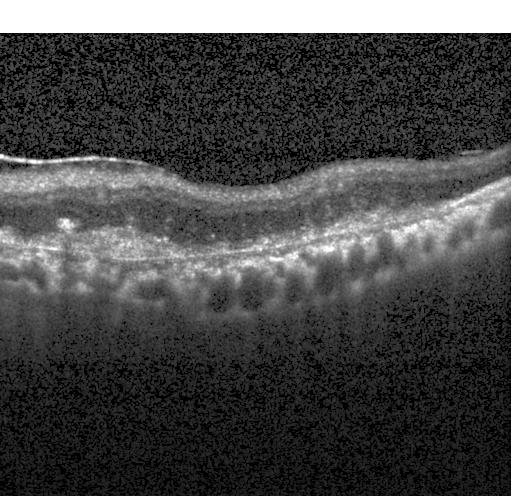

Acquired on a Heidelberg Spectralis. OCT B-scan.
Impression: choroidal neovascularization.